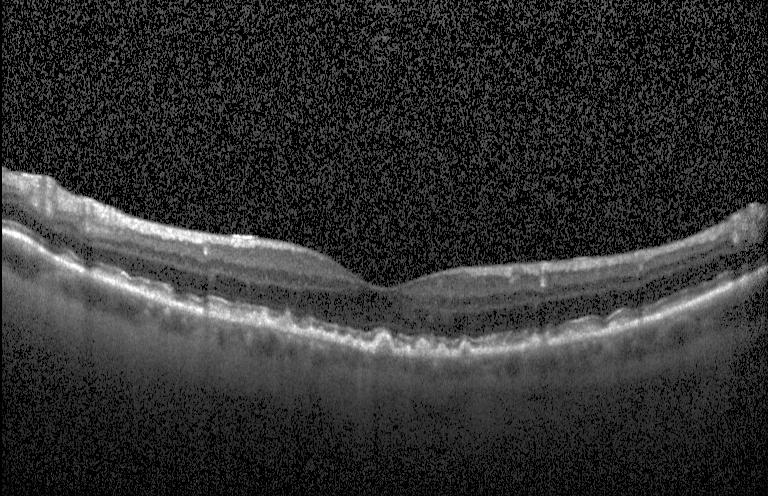 Macular OCT: drusen.